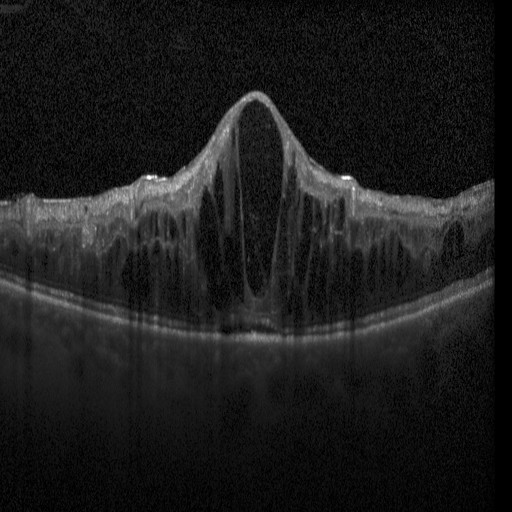
Retinal OCT cross-section. Spectral-domain OCT. Heidelberg Spectralis OCT system. Centered on the fovea.
Diabetic macular edema.